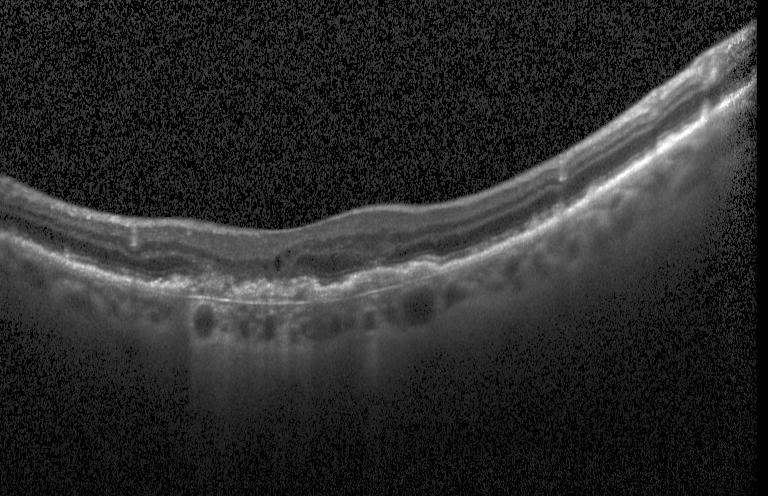
Instrument: Heidelberg Spectralis, OCT B-scan, spectral-domain OCT.
A choroidal neovascular membrane.